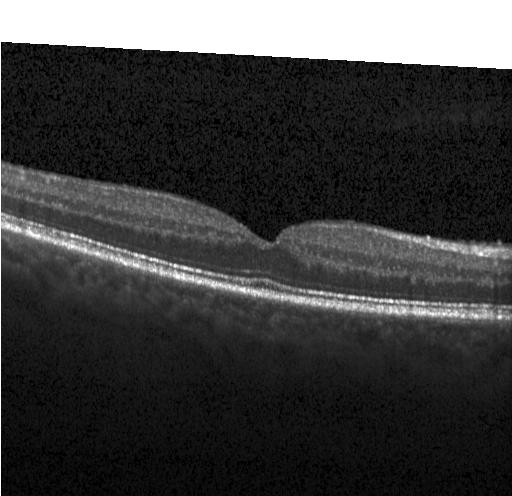 OCT finding: no choroidal neovascularization, no diabetic macular edema, and no drusen.